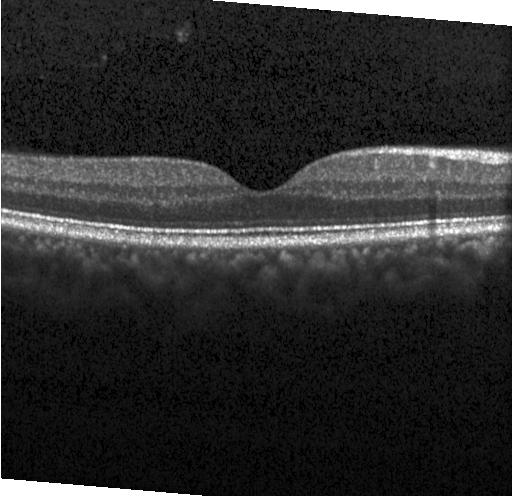 Retinal OCT cross-section. Heidelberg Spectralis. Through the macula — Diagnosis: neither choroidal neovascularization, diabetic macular edema, nor drusen.